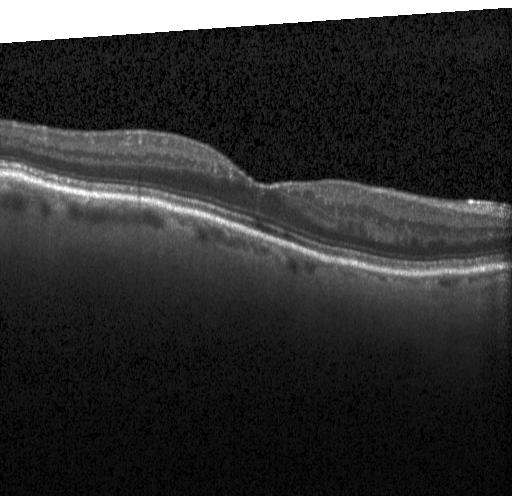

Instrument: Heidelberg Spectralis. Optical coherence tomography B-scan
Impression: neither CNV, DME, nor drusen.